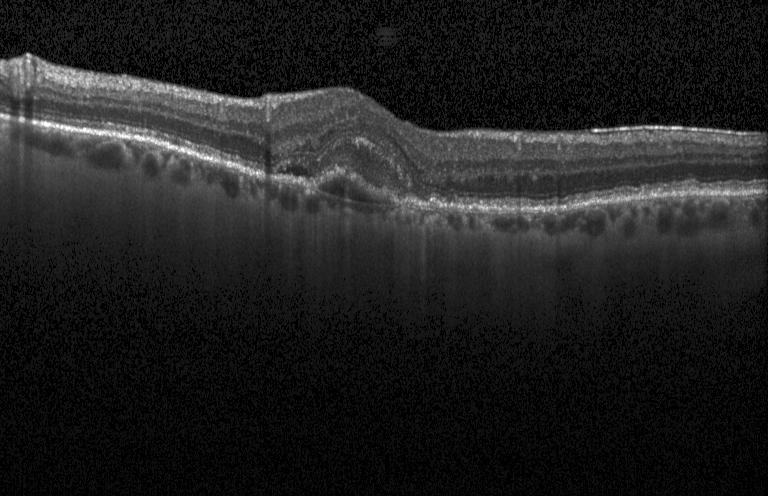 Finding: CNV.